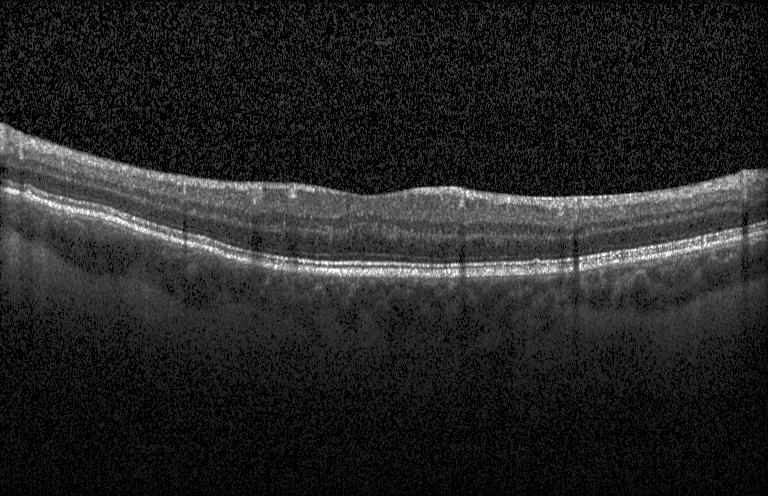
OCT line scan.
Macular OCT: no choroidal neovascularization, no diabetic macular edema, and no drusen.